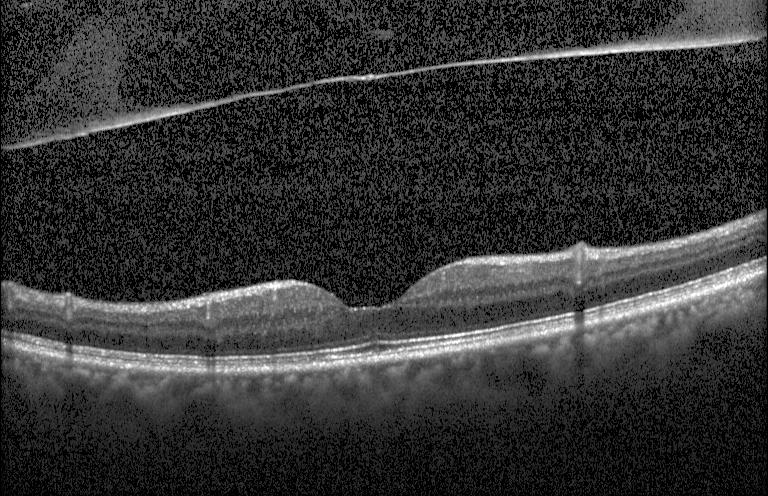

Optical coherence tomography scan — Macular OCT: no choroidal neovascularization, no diabetic macular edema, and no drusen.